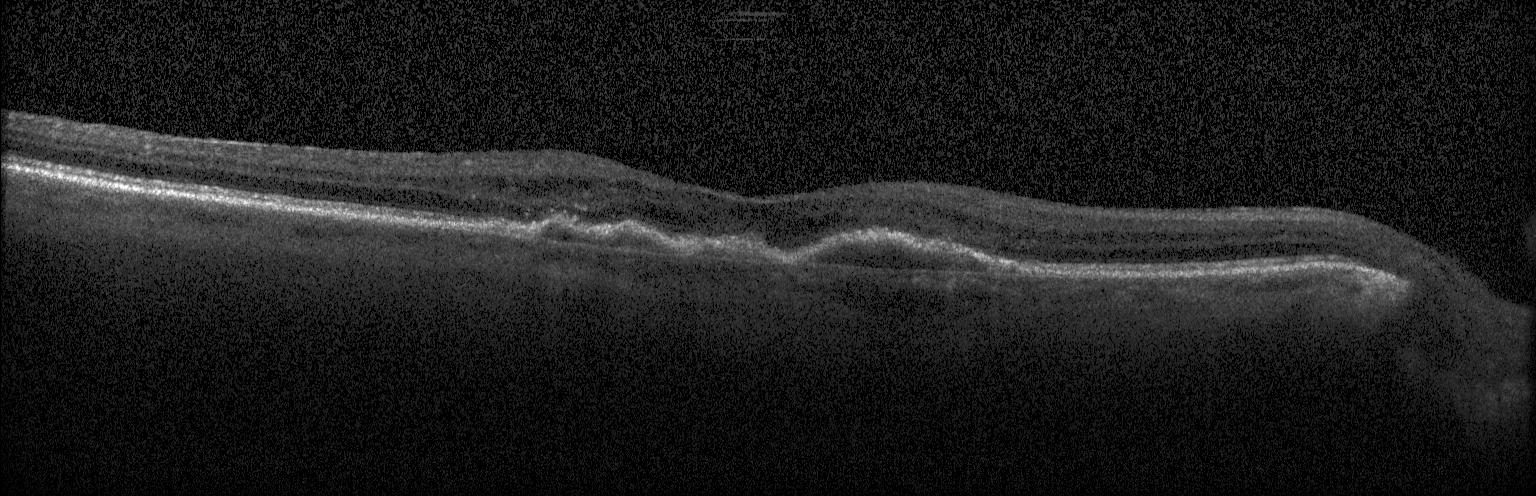

Impression: CNV.